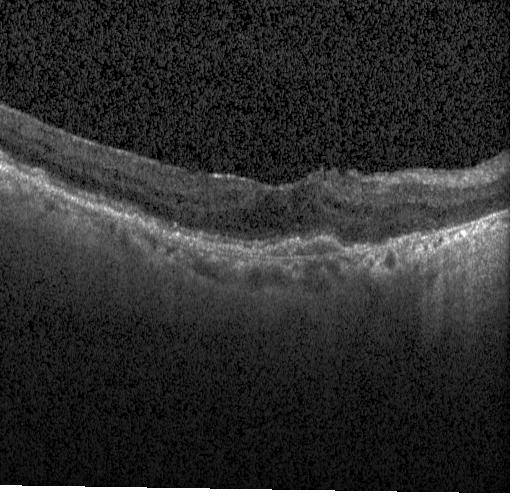
Finding: a choroidal neovascular membrane.